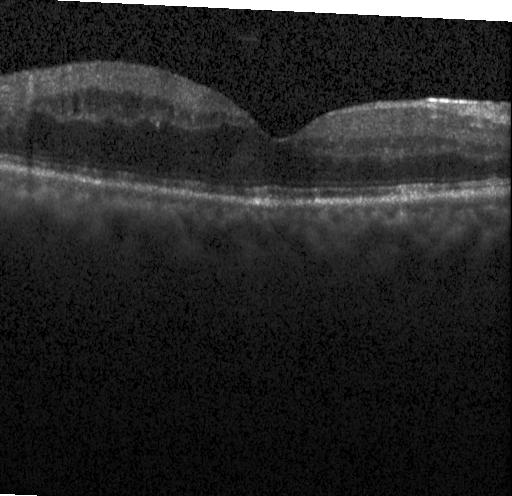
Centered on the fovea; retinal OCT cross-section — DME.